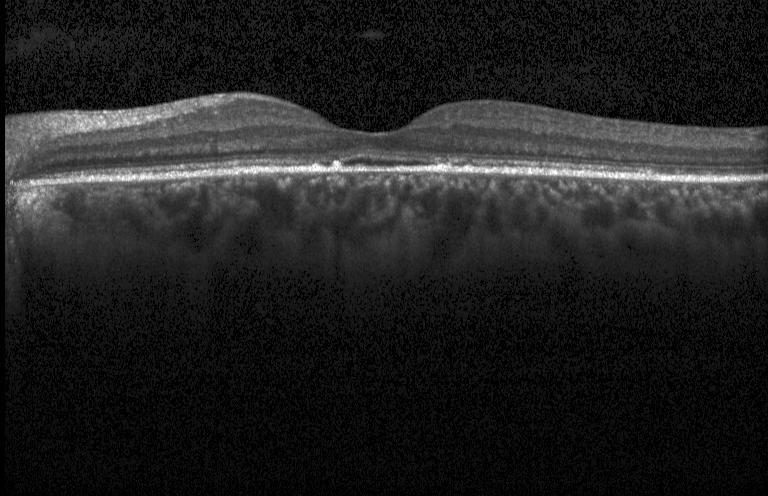 Dx: no evidence of CNV, DME, or drusen.